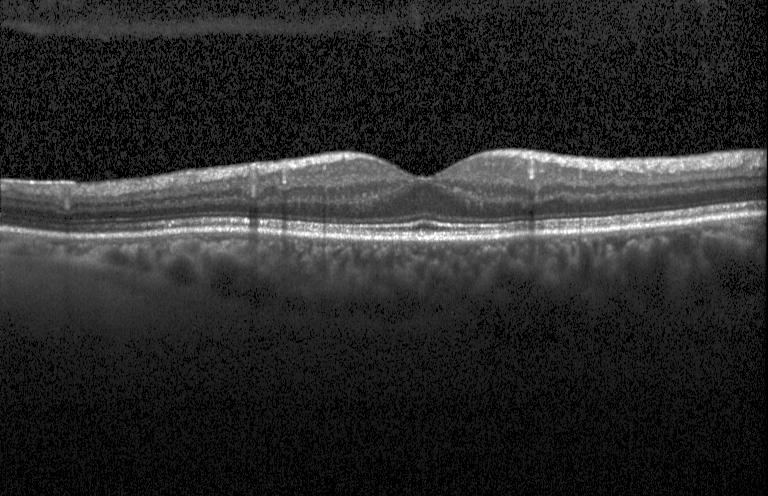
Macular scan · OCT line scan · spectral-domain optical coherence tomography.
Dx: neither choroidal neovascularization, diabetic macular edema, nor drusen.